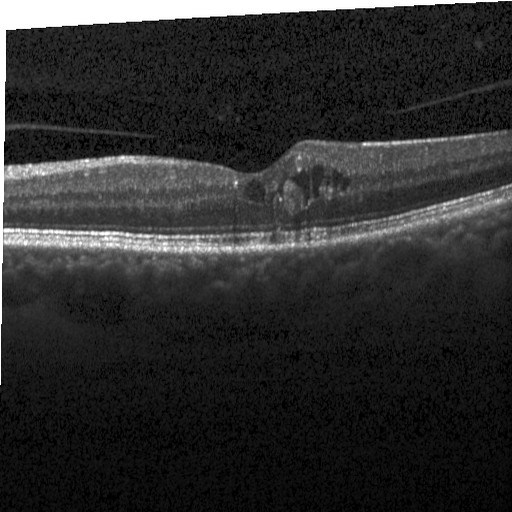 Optical coherence tomography scan.
Assessment: diabetic macular edema (DME).